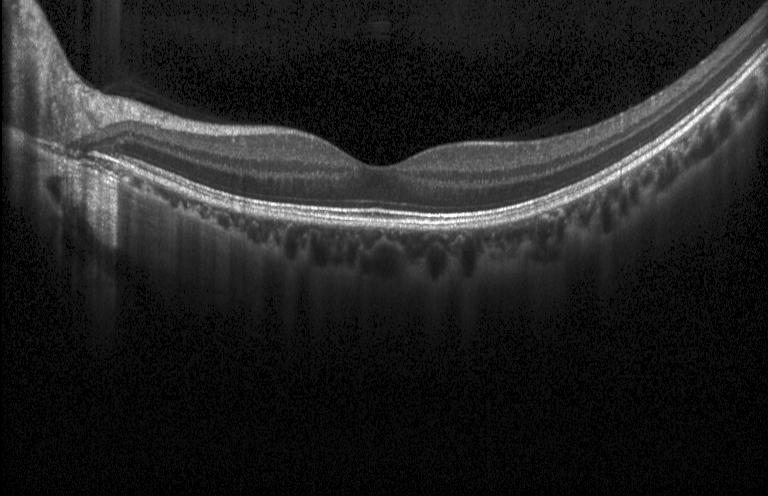

Centered on the fovea, spectral-domain OCT, retinal OCT cross-section, acquired on a Heidelberg Spectralis — The scan shows neither CNV, DME, nor drusen.